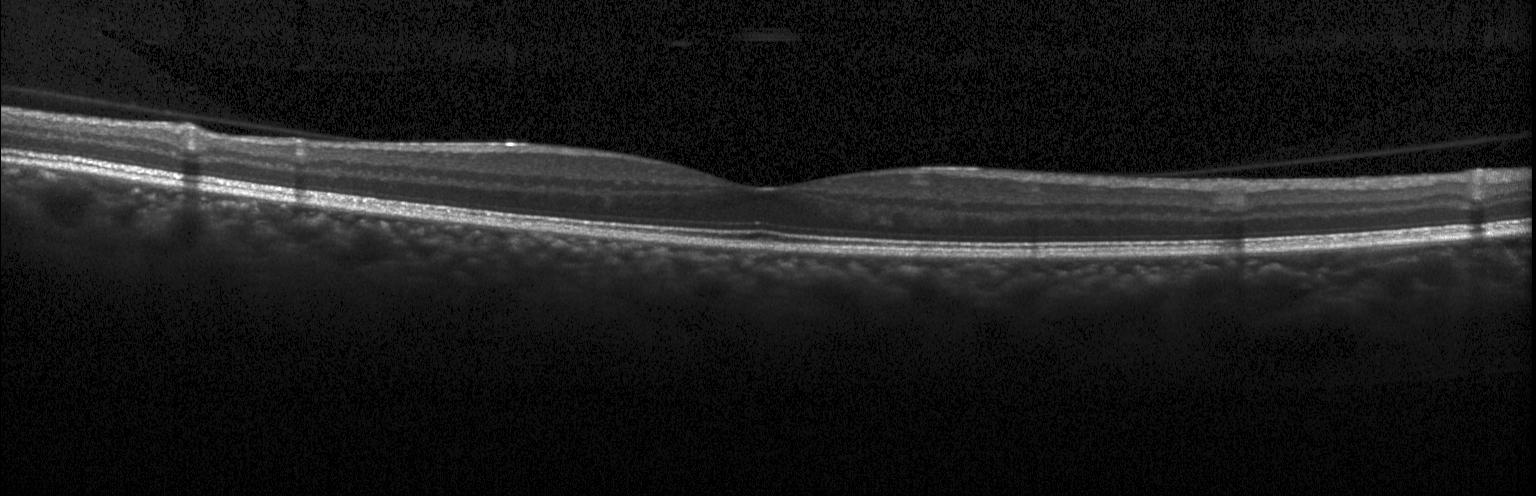

Diagnosis: no choroidal neovascularization, no diabetic macular edema, and no drusen.